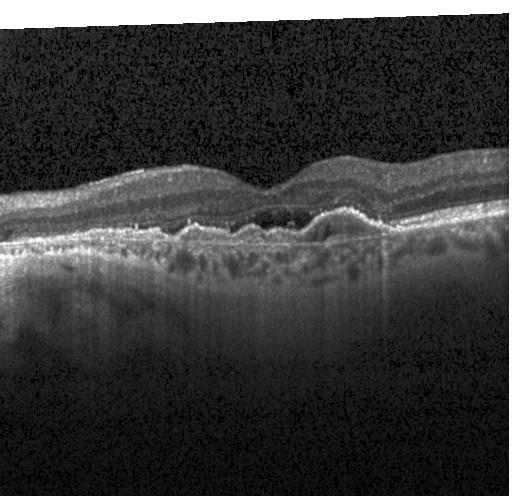

OCT line scan.
Diagnosis: a choroidal neovascular membrane.